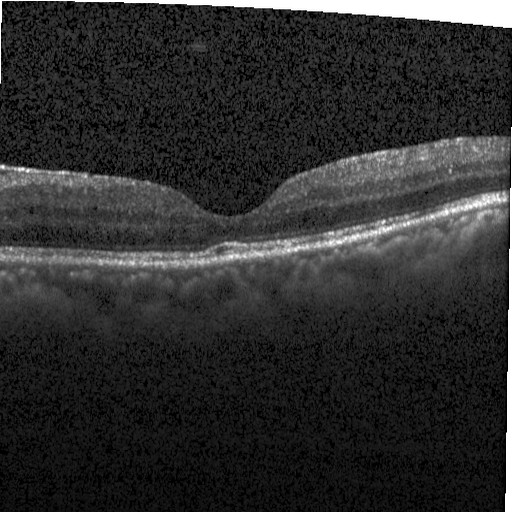 Spectral-domain optical coherence tomography · OCT B-scan · Heidelberg Spectralis. Diagnosis: diabetic macular edema (DME).